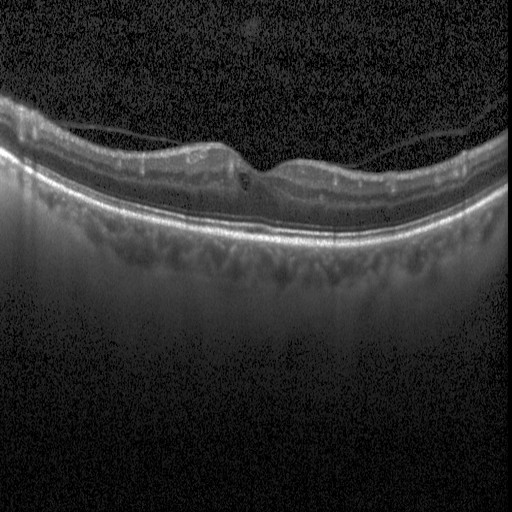

Retinal OCT cross-section
Assessment: DME.